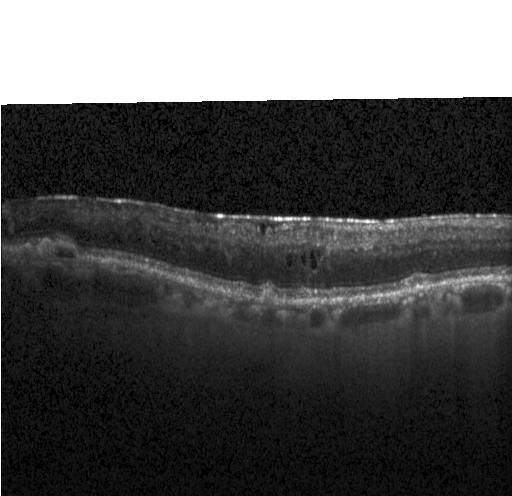
Diagnosis: a choroidal neovascular membrane.